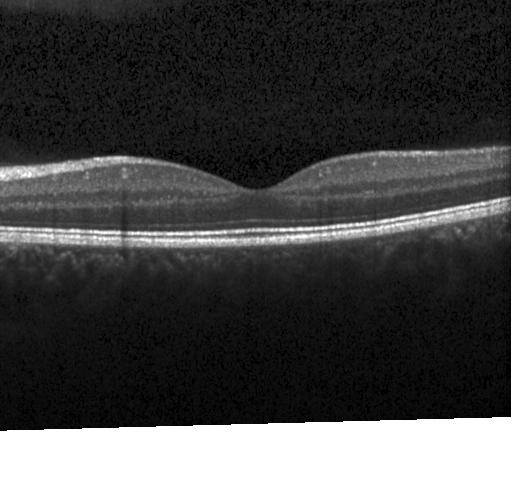

Diagnosis: no CNV, no DME, and no drusen.